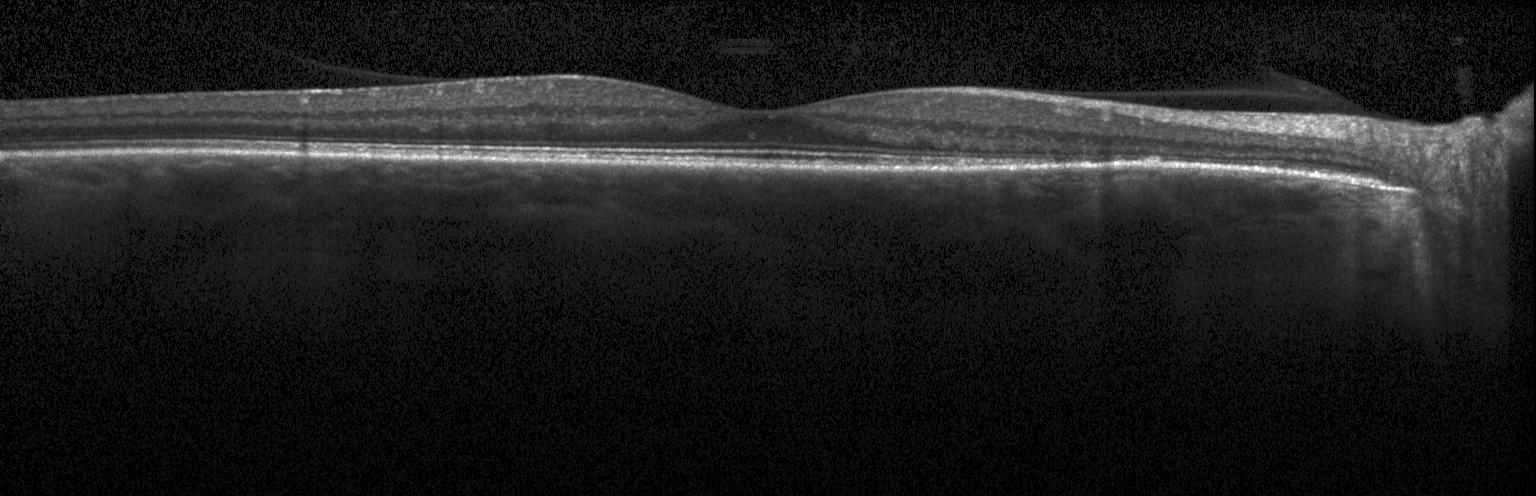
Optical coherence tomography B-scan · through the macula. Macular OCT: no evidence of choroidal neovascularization, diabetic macular edema, or drusen.